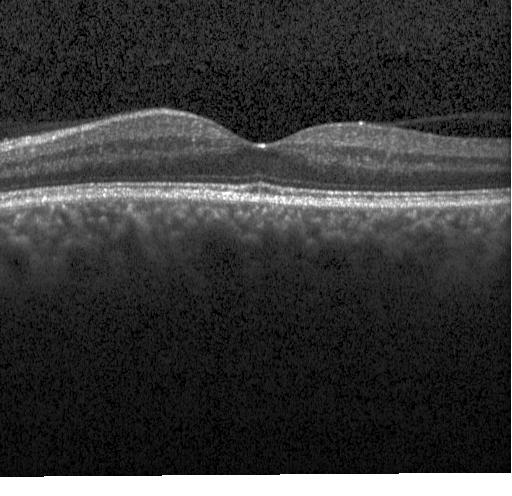

Assessment: neither CNV, DME, nor drusen.